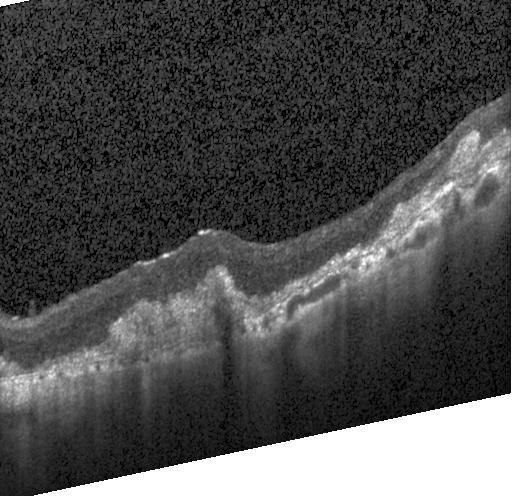

OCT finding: CNV.